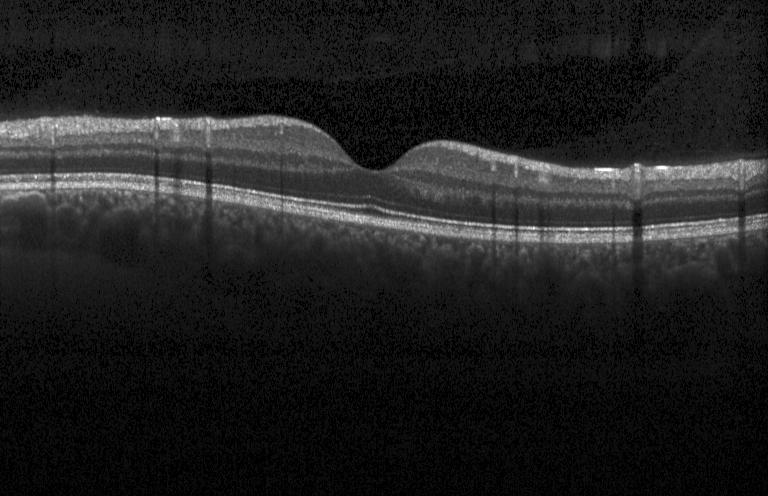

Retinal OCT B-scan. Instrument: Heidelberg Spectralis. Spectral-domain OCT.
OCT finding: neither choroidal neovascularization, diabetic macular edema, nor drusen.